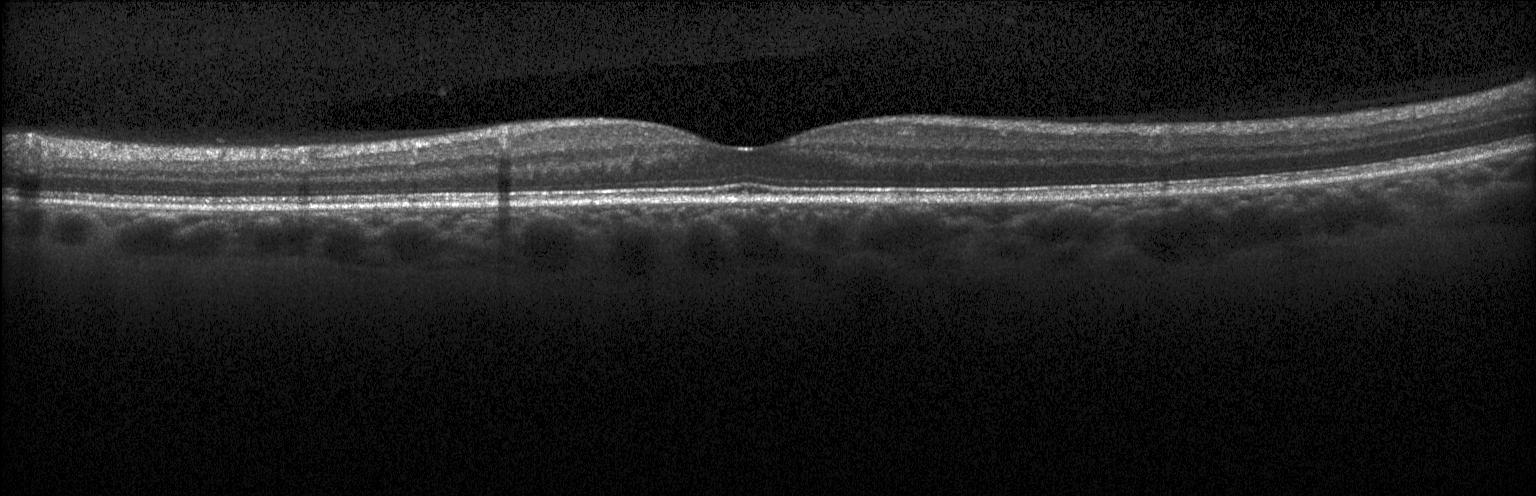
Optical coherence tomography scan, Heidelberg Spectralis, SD-OCT.
Assessment: no choroidal neovascularization, diabetic macular edema, or drusen.